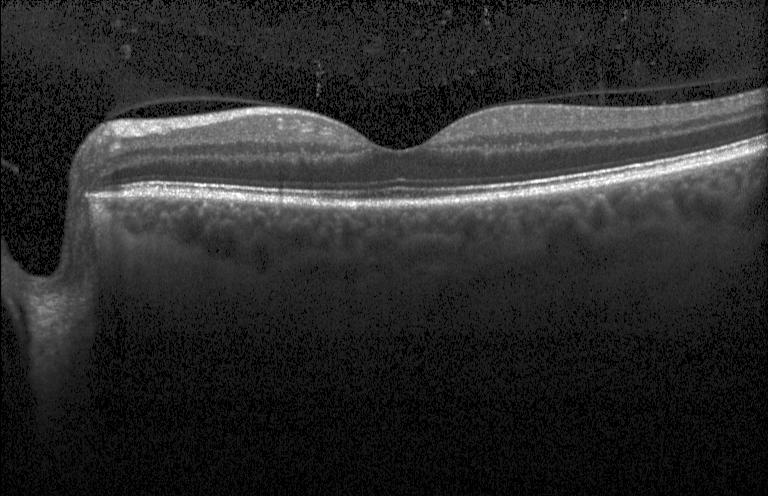 OCT line scan. Horizontal scan through the fovea. Heidelberg Spectralis OCT system. This B-scan demonstrates no CNV, no DME, and no drusen.